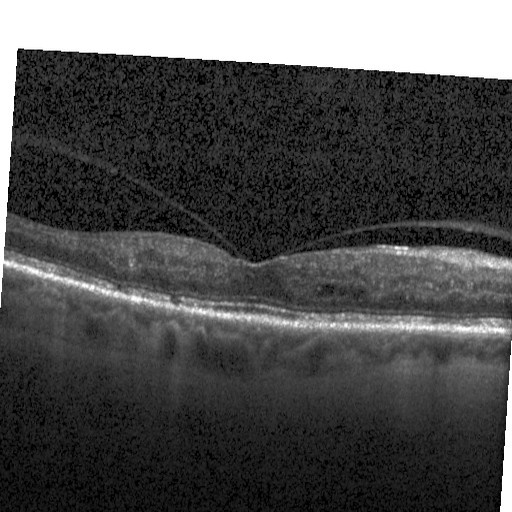

Acquired on a Heidelberg Spectralis; OCT line scan; spectral-domain OCT.
Assessment: diabetic macular edema.